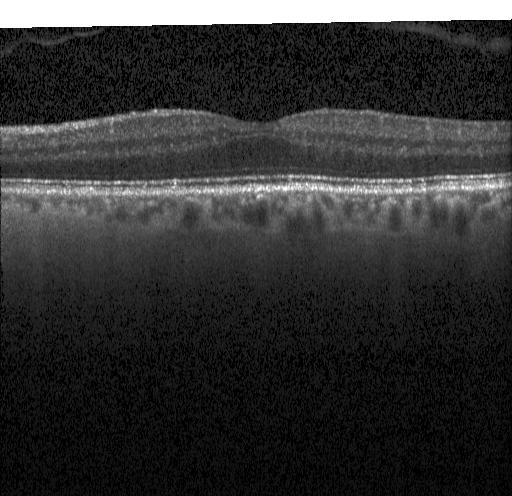
Centered on the fovea. Spectral-domain optical coherence tomography. Retinal OCT cross-section. Instrument: Heidelberg Spectralis — Dx: no evidence of choroidal neovascularization, diabetic macular edema, or drusen.